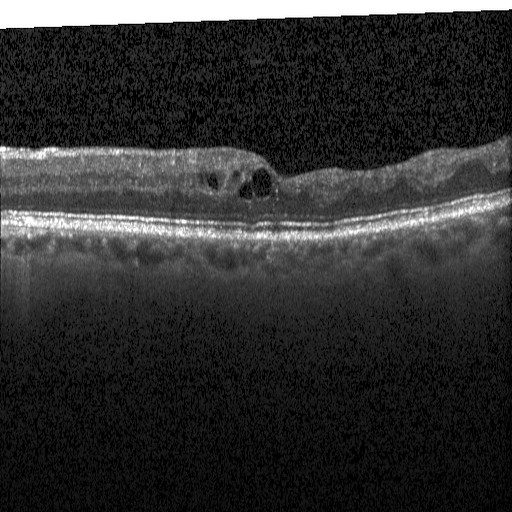

Diagnosis: DME.